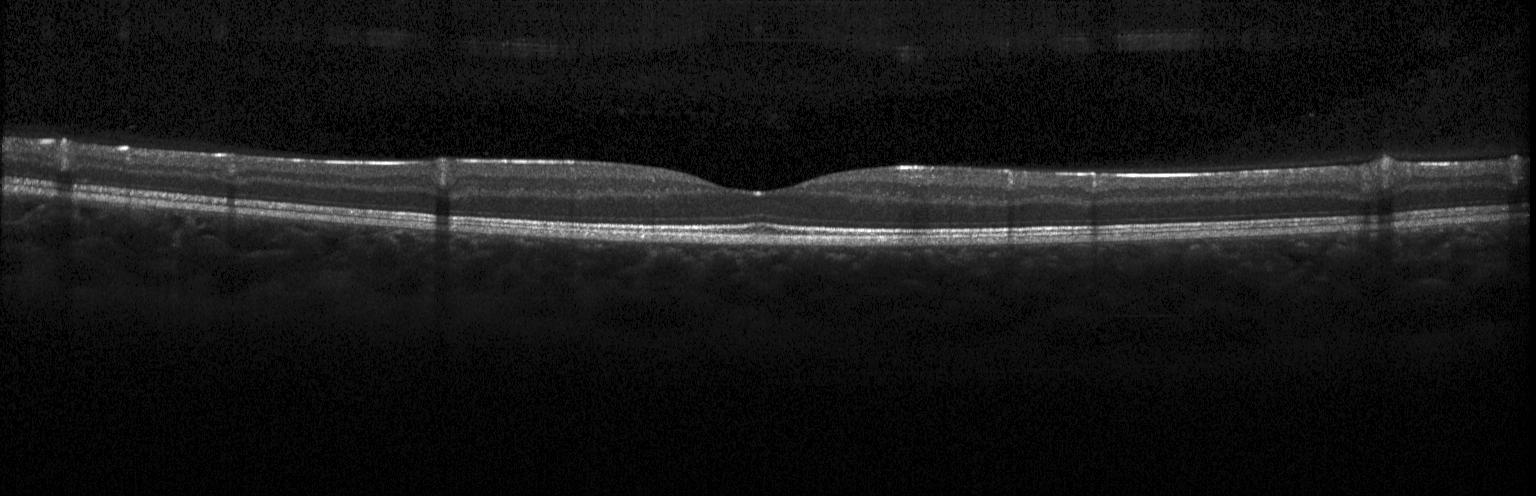
Optical coherence tomography scan — Diagnosis: neither CNV, DME, nor drusen.